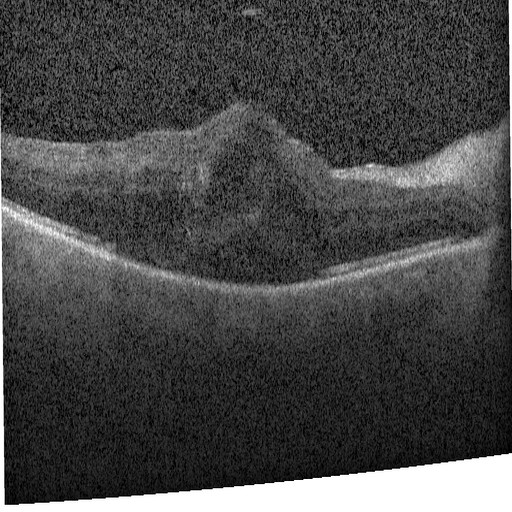

Retinal OCT B-scan; through the macula. Diagnosis: diabetic macular edema.